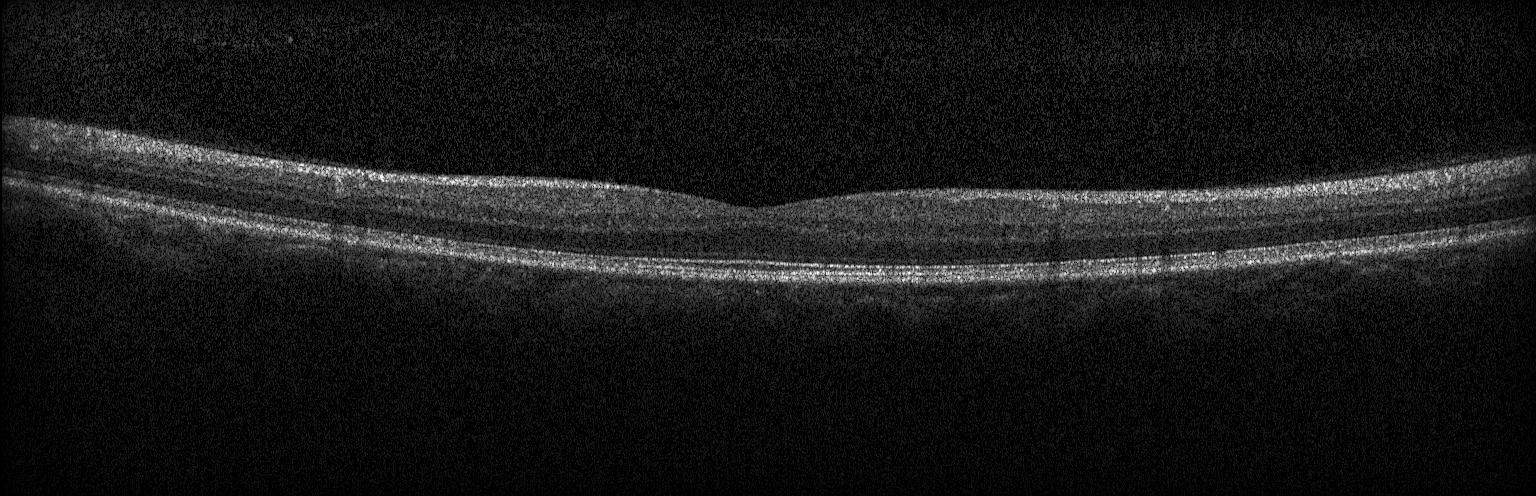

Optical coherence tomography scan. Neither CNV, DME, nor drusen.